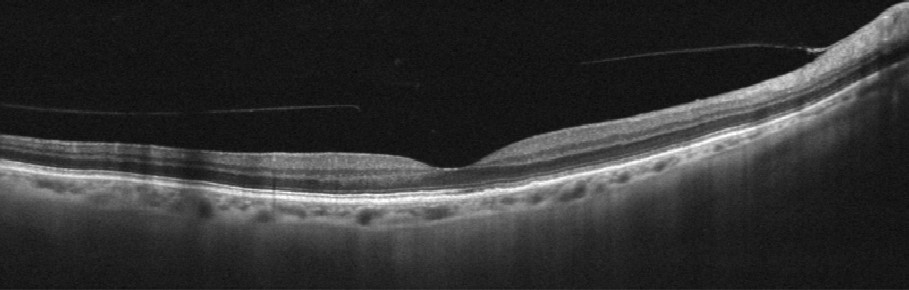 This B-scan demonstrates age-related macular degeneration.